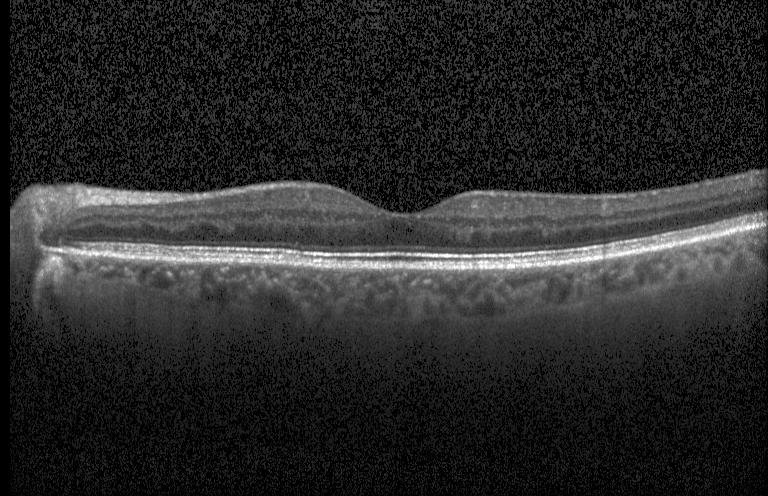
Spectral-domain OCT · instrument: Heidelberg Spectralis · optical coherence tomography scan
Dx: neither CNV, DME, nor drusen.